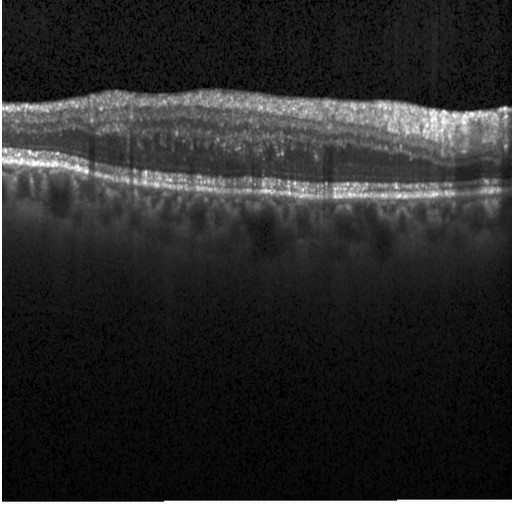

Macular OCT: diabetic macular edema (DME).